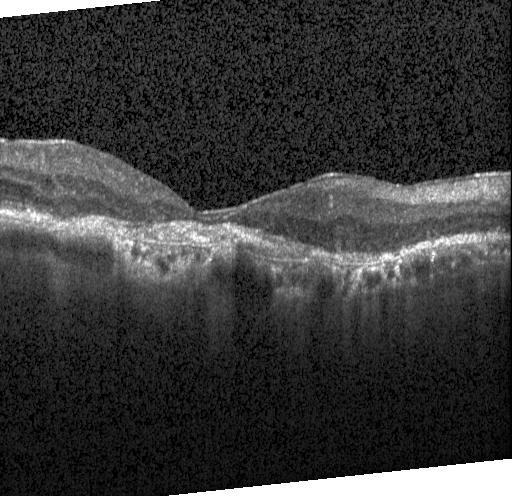

Retinal OCT cross-section.
OCT finding: a choroidal neovascular membrane.